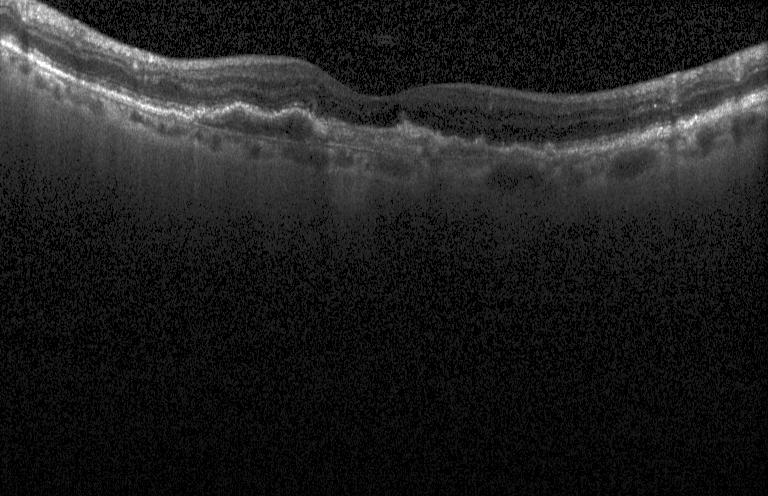

Retinal OCT cross-section; acquired on a Heidelberg Spectralis — Assessment: a choroidal neovascular membrane.